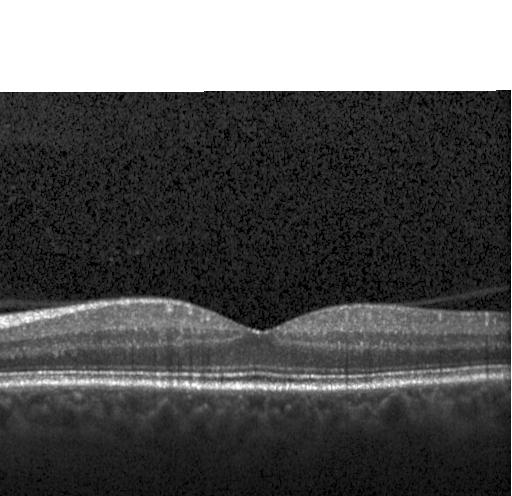 OCT finding: no evidence of choroidal neovascularization, diabetic macular edema, or drusen.